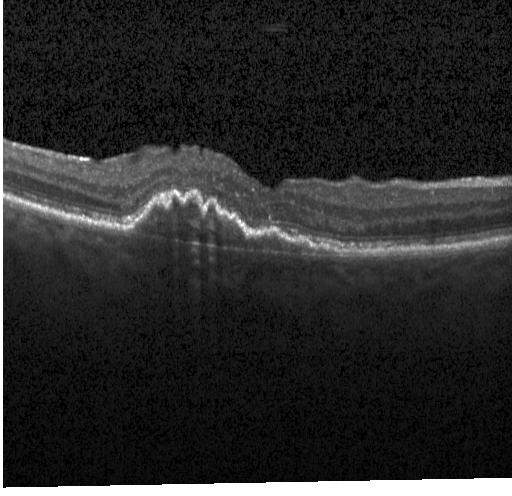
Heidelberg Spectralis OCT system, centered on the fovea, spectral-domain optical coherence tomography, OCT line scan. Diagnosis: CNV.